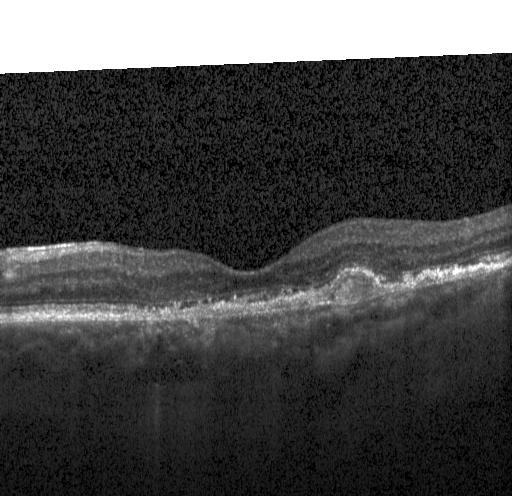
Spectral-domain OCT B-scan: choroidal neovascularization (CNV).